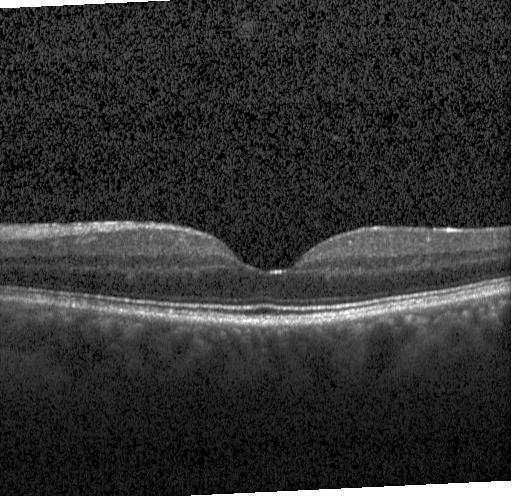
Optical coherence tomography B-scan · spectral-domain optical coherence tomography.
OCT finding: no evidence of choroidal neovascularization, diabetic macular edema, or drusen.